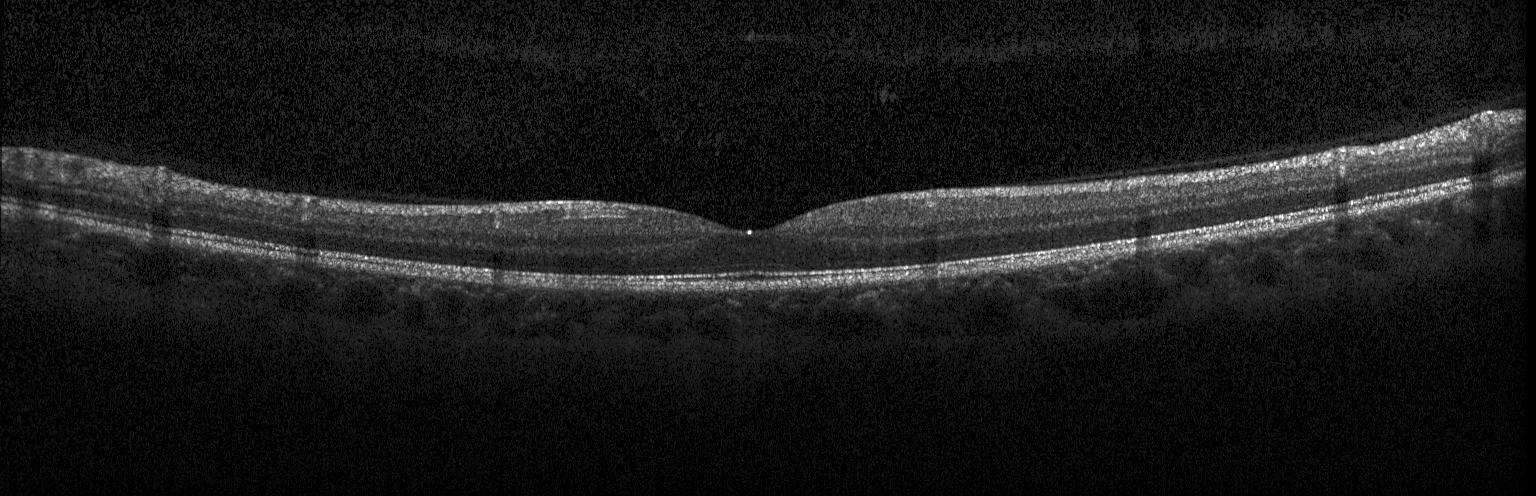

Spectral-domain OCT B-scan: no CNV, no DME, and no drusen.